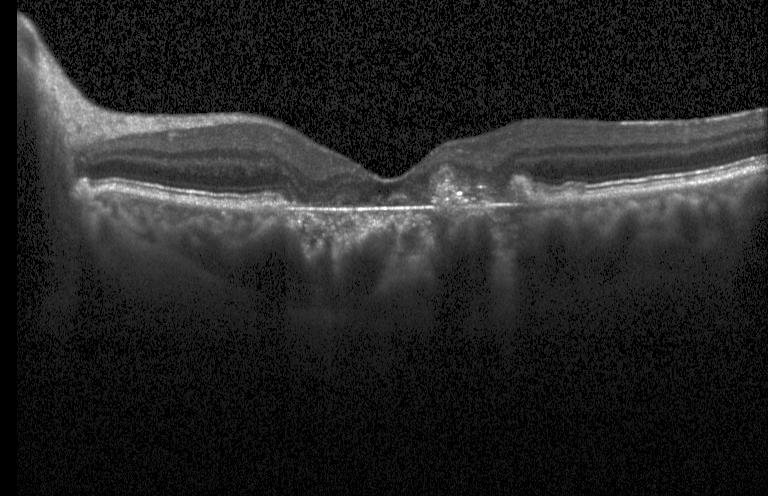 Instrument: Heidelberg Spectralis · spectral-domain OCT · fovea-centered · optical coherence tomography scan.
Macular OCT: a choroidal neovascular membrane.